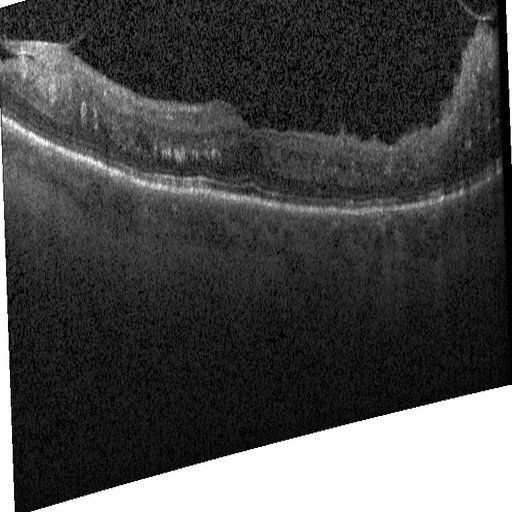

Finding: diabetic macular edema.